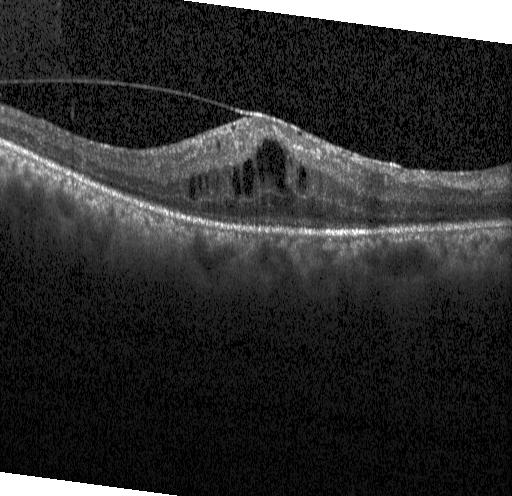

Assessment: diabetic macular edema (DME).